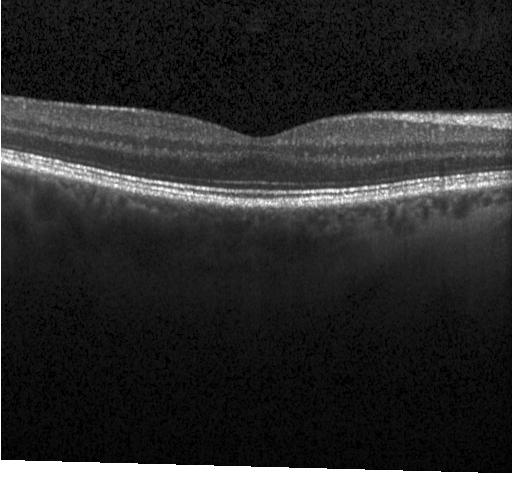

Retinal OCT cross-section. Diagnosis: no evidence of choroidal neovascularization, diabetic macular edema, or drusen.